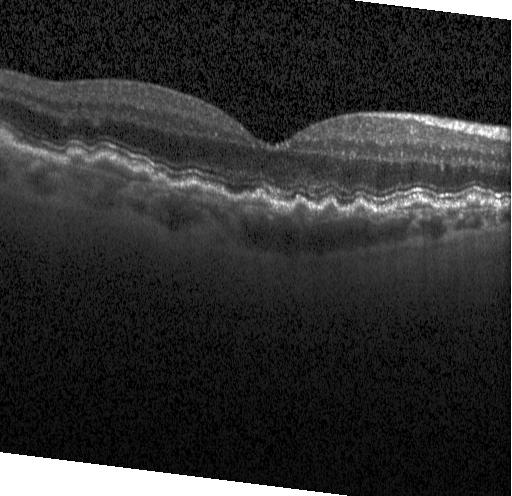
Dx: sub-RPE drusenoid deposits.